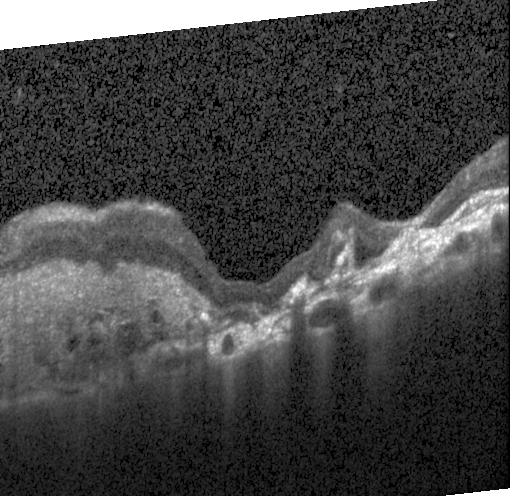
SD-OCT. Macular scan. OCT B-scan
This B-scan demonstrates choroidal neovascularization.